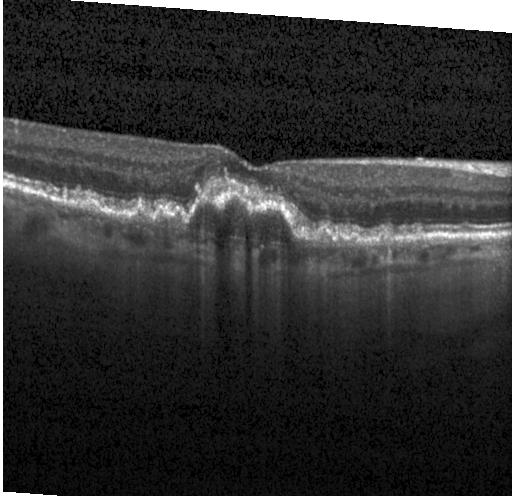 SD-OCT; Heidelberg Spectralis; optical coherence tomography scan; macular scan.
OCT finding: a choroidal neovascular membrane.